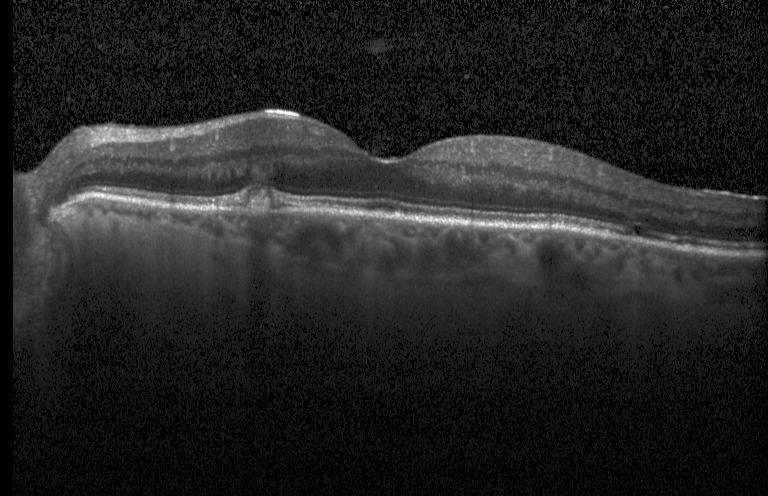 Macular OCT demonstrating multiple drusen.